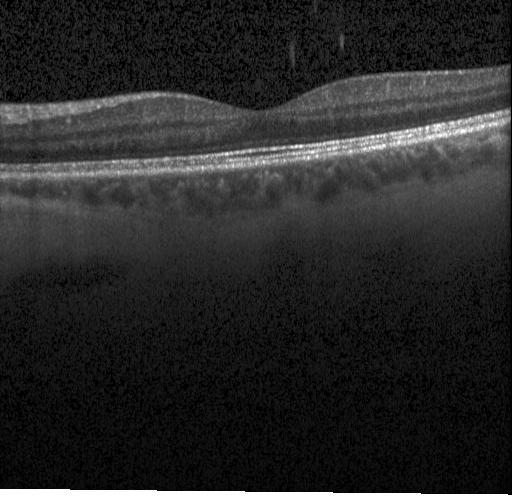 Through the macula; optical coherence tomography scan — This B-scan demonstrates no evidence of choroidal neovascularization, diabetic macular edema, or drusen.